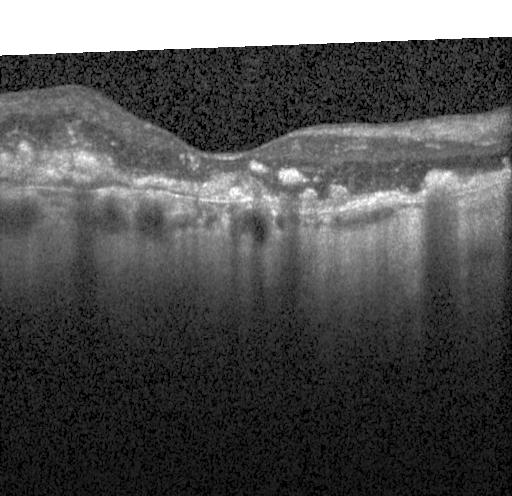 SD-OCT. Heidelberg Spectralis OCT system. OCT line scan. Centered on the fovea.
Finding: choroidal neovascularization (CNV).